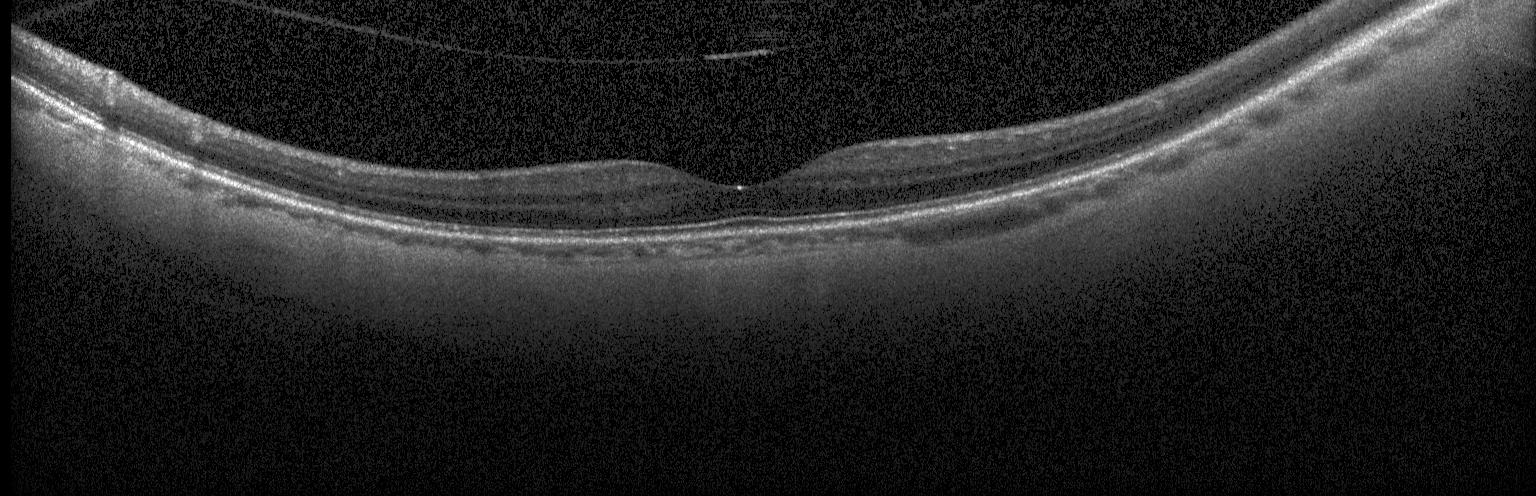
OCT line scan. Through the macula. Heidelberg Spectralis.
Diagnosis: no choroidal neovascularization, no diabetic macular edema, and no drusen.